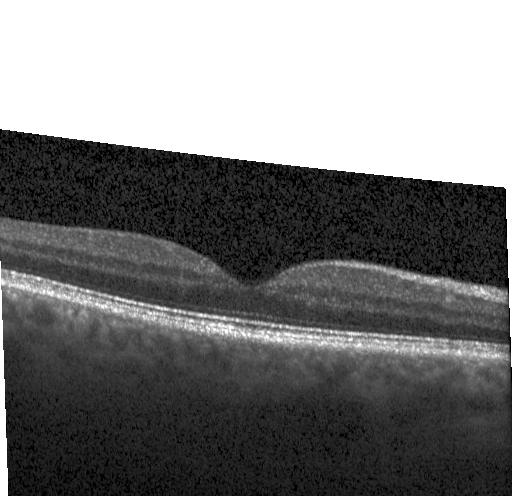 OCT line scan. Diagnosis: neither choroidal neovascularization, diabetic macular edema, nor drusen.